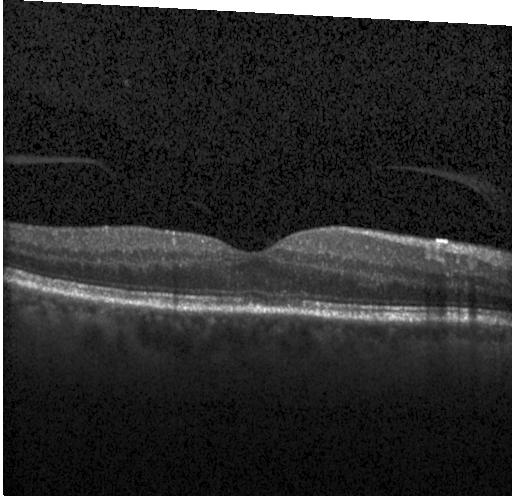 Heidelberg Spectralis · centered on the fovea · SD-OCT · OCT line scan — OCT finding: no choroidal neovascularization, no diabetic macular edema, and no drusen.